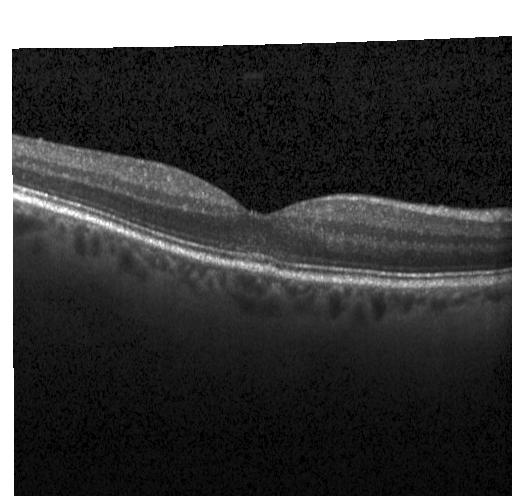
Spectral-domain OCT · Heidelberg Spectralis OCT system · retinal OCT cross-section. Impression: no choroidal neovascularization, diabetic macular edema, or drusen.